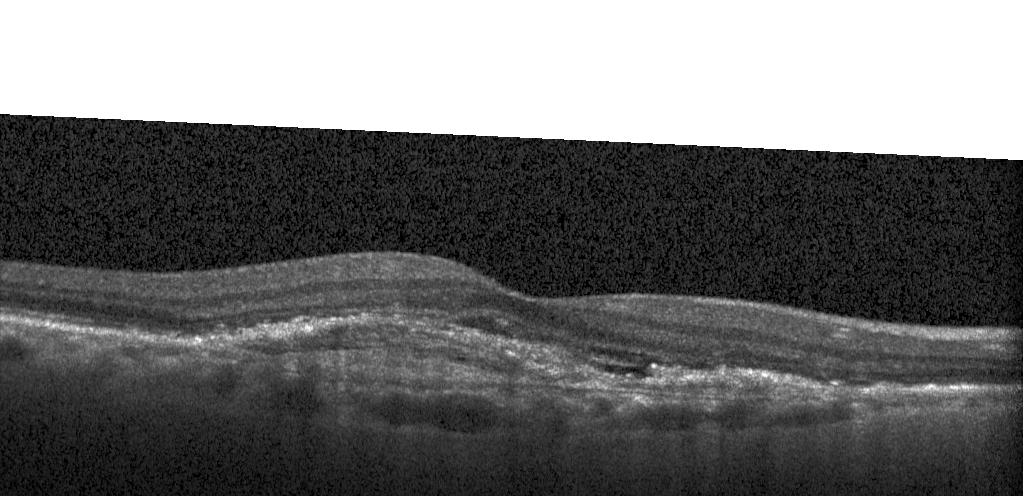

The scan shows CNV.